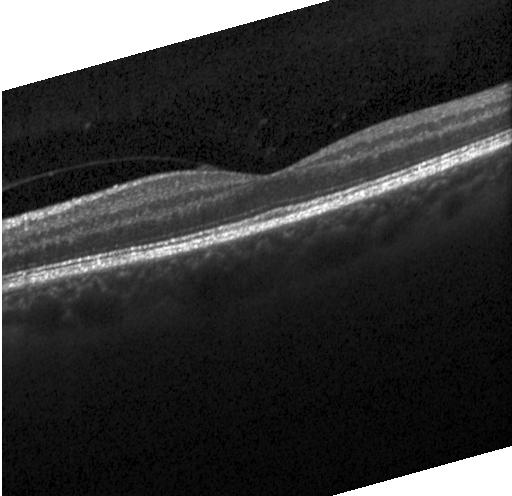
Retinal OCT cross-section
Impression: neither CNV, DME, nor drusen.